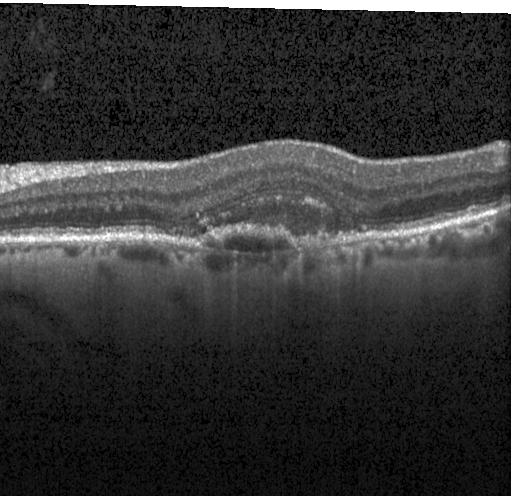
Optical coherence tomography B-scan. Heidelberg Spectralis OCT system. This B-scan demonstrates a choroidal neovascular membrane.